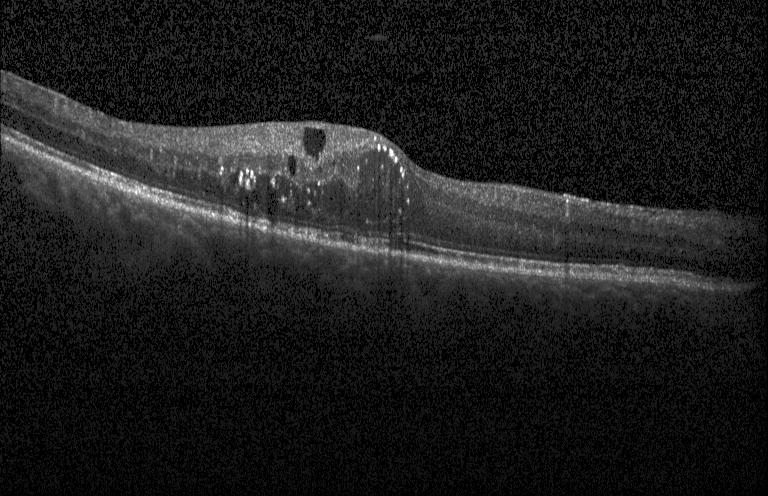

Spectral-domain OCT B-scan: diabetic macular edema.